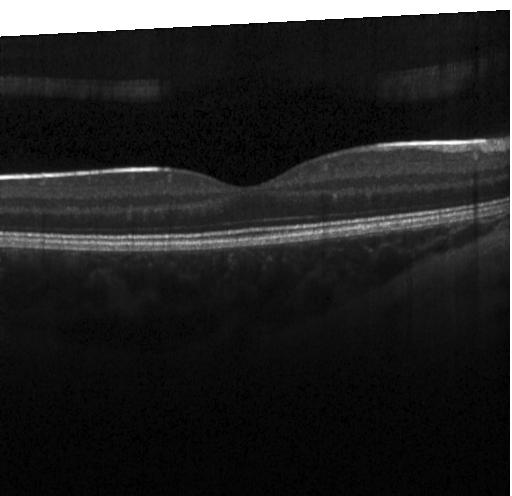 OCT B-scan showing no choroidal neovascularization, no diabetic macular edema, and no drusen.